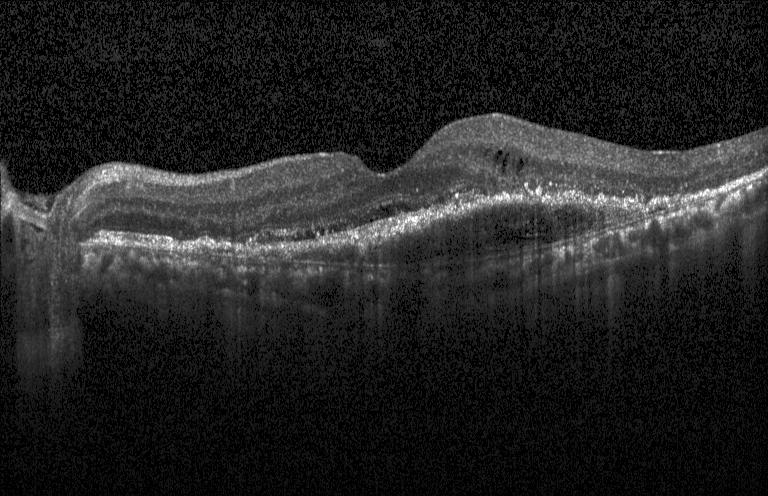

Finding: CNV.